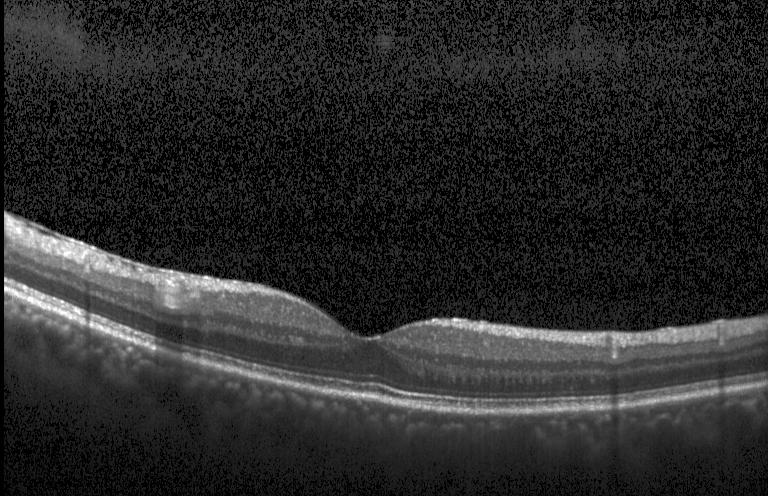 OCT finding: no evidence of choroidal neovascularization, diabetic macular edema, or drusen.